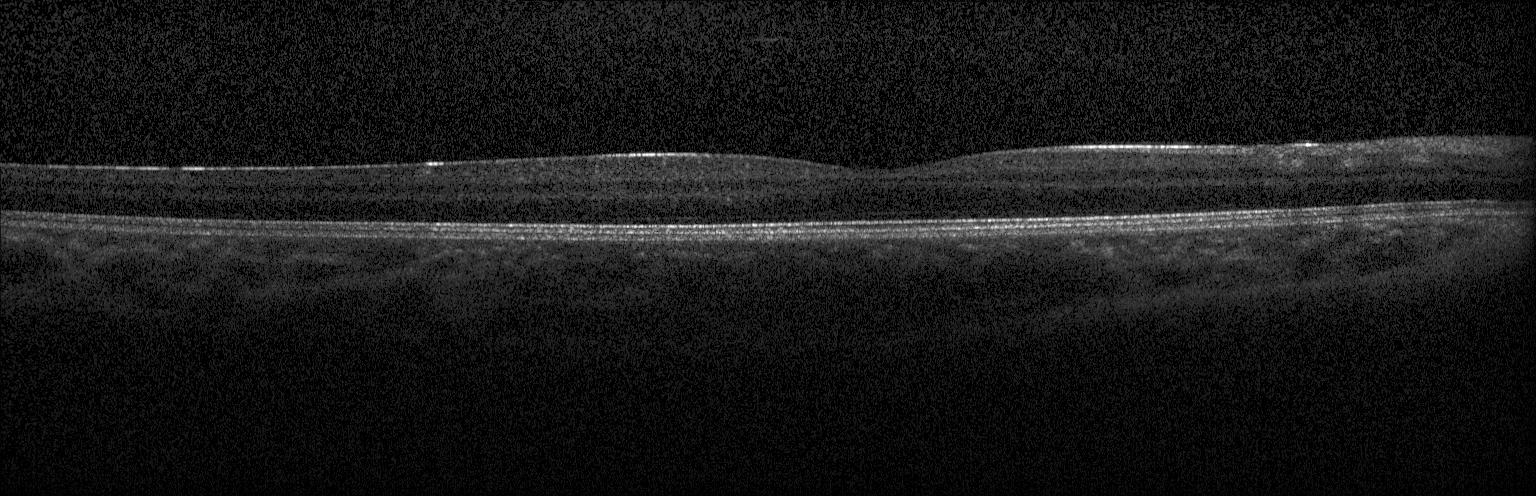 Optical coherence tomography B-scan — Finding: no evidence of choroidal neovascularization, diabetic macular edema, or drusen.